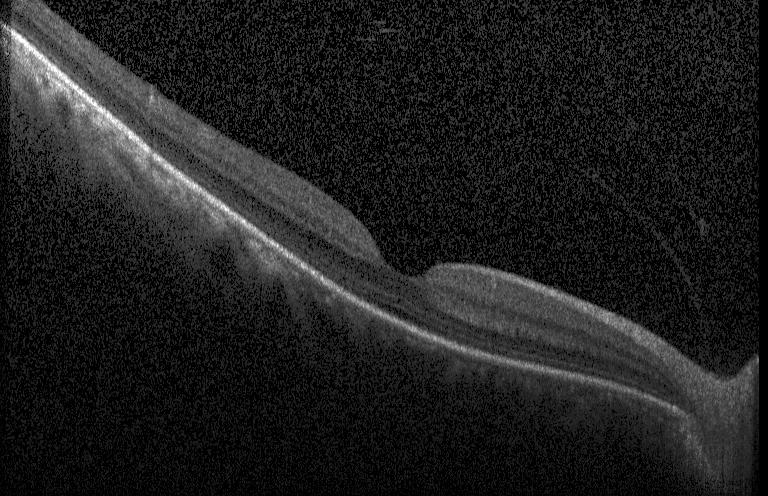
Finding: no choroidal neovascularization, no diabetic macular edema, and no drusen.